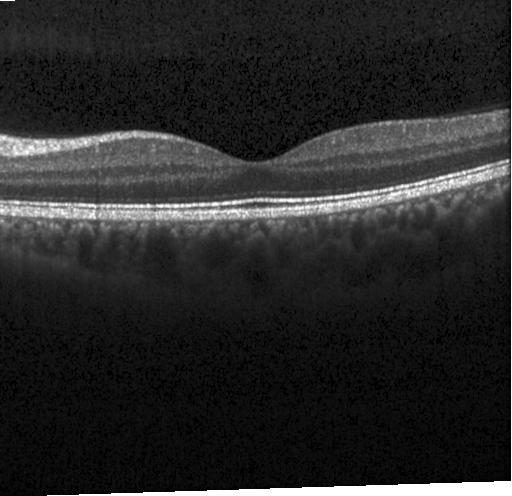

Spectral-domain optical coherence tomography · acquired on a Heidelberg Spectralis · optical coherence tomography scan.
Assessment: no evidence of choroidal neovascularization, diabetic macular edema, or drusen.